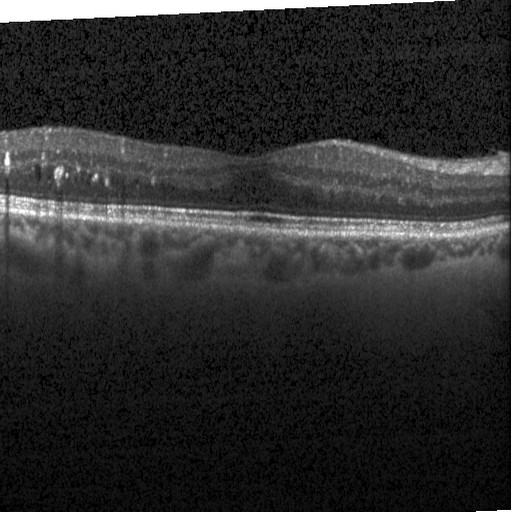 Spectral-domain OCT. Heidelberg Spectralis. OCT B-scan.
Finding: diabetic macular edema.